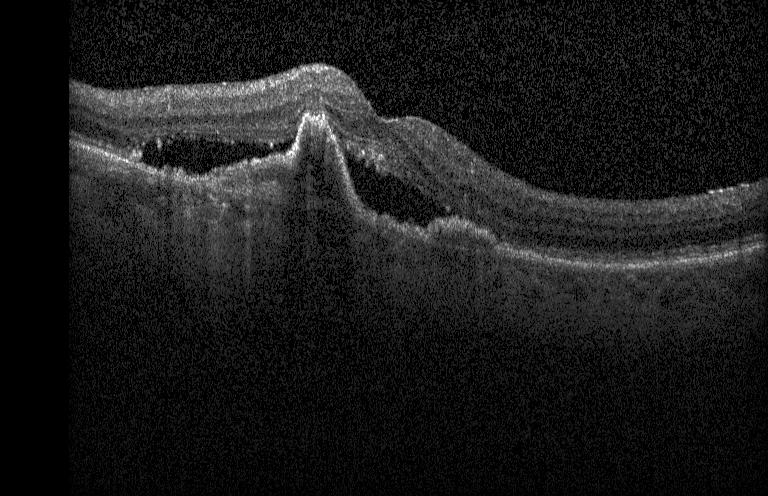
OCT B-scan showing CNV.